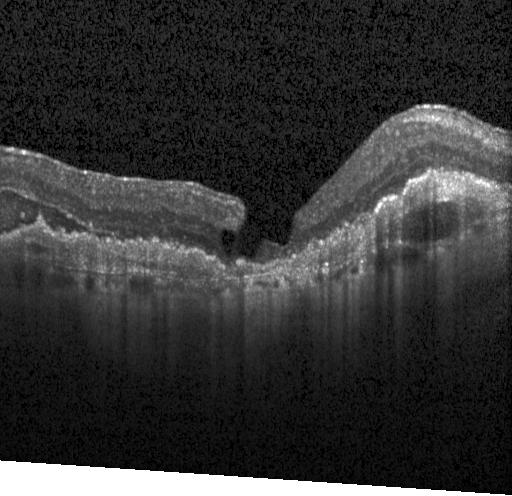 Diagnosis: a choroidal neovascular membrane.